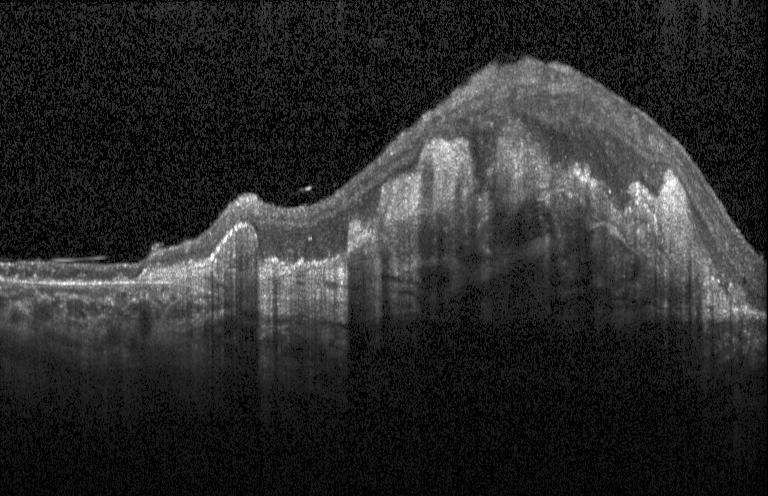 Spectral-domain OCT. Retinal OCT B-scan. Acquired on a Heidelberg Spectralis.
Assessment: a choroidal neovascular membrane.